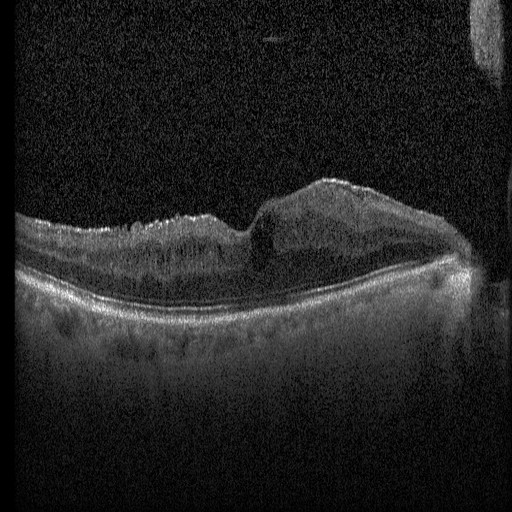
Fovea-centered · optical coherence tomography scan · Heidelberg Spectralis OCT system.
Impression: diabetic macular edema.